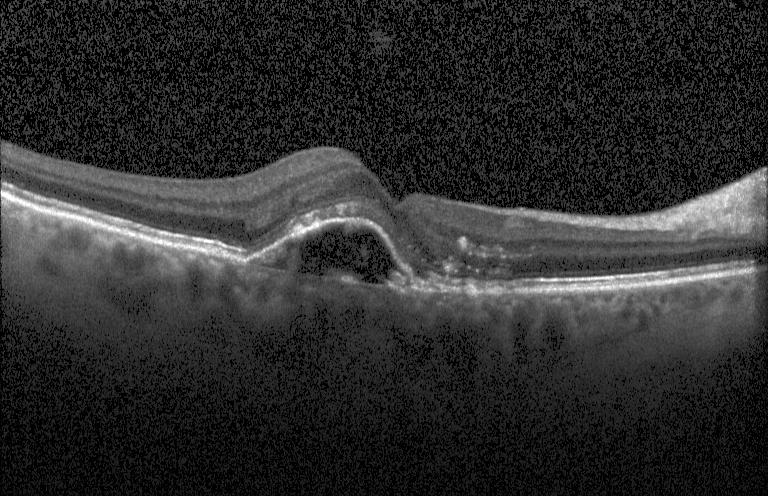
Optical coherence tomography B-scan, spectral-domain OCT — Impression: CNV.